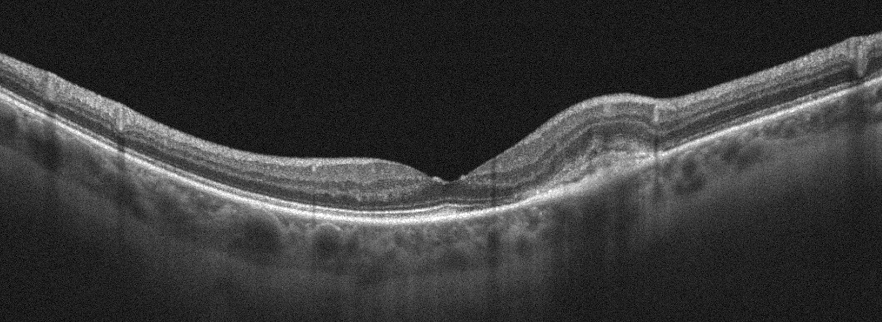 Finding: age-related macular degeneration.